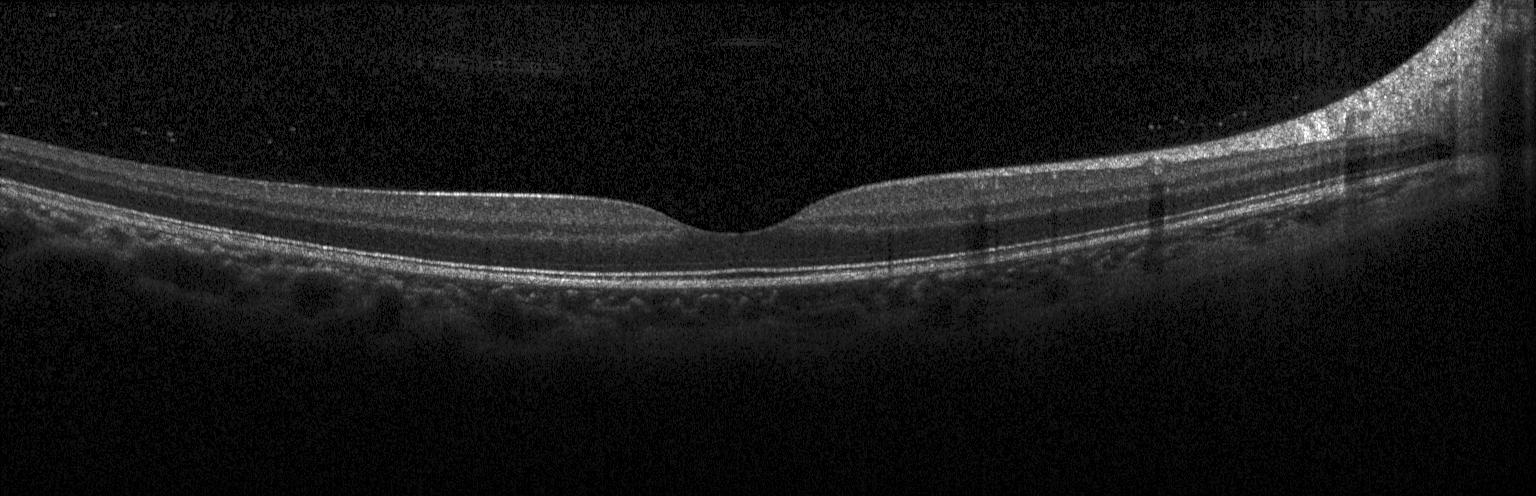
Retinal OCT cross-section, instrument: Heidelberg Spectralis, horizontal scan through the fovea
The scan shows neither CNV, DME, nor drusen.